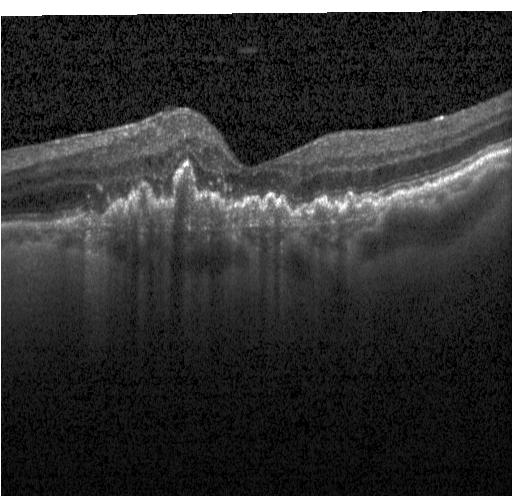 A choroidal neovascular membrane.